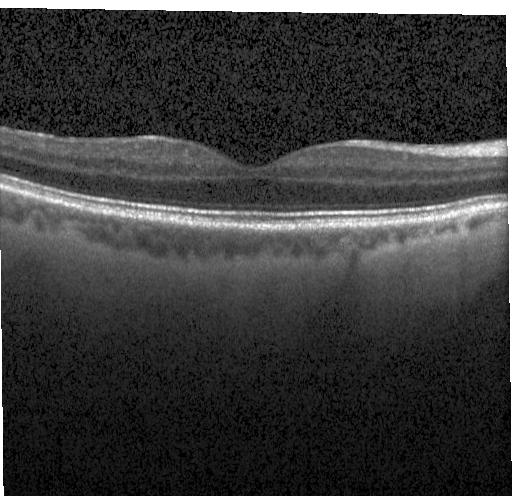

OCT line scan, acquired on a Heidelberg Spectralis, centered on the fovea
Macular OCT: no choroidal neovascularization, diabetic macular edema, or drusen.